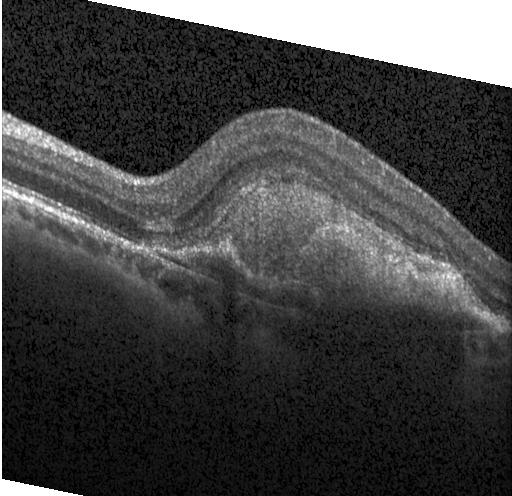

Retinal OCT cross-section. Through the macula. OCT finding: CNV.